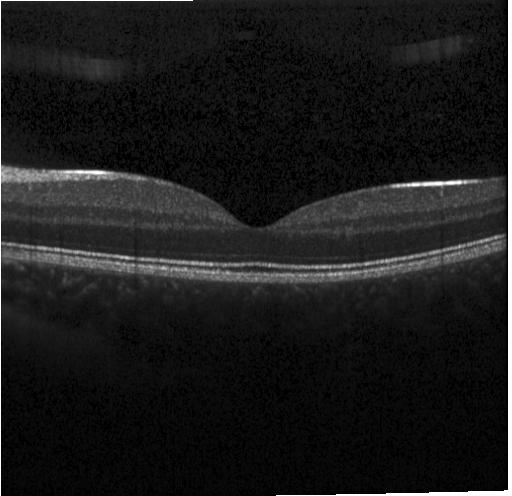

Optical coherence tomography B-scan; SD-OCT; Heidelberg Spectralis; through the macula
Assessment: no choroidal neovascularization, no diabetic macular edema, and no drusen.